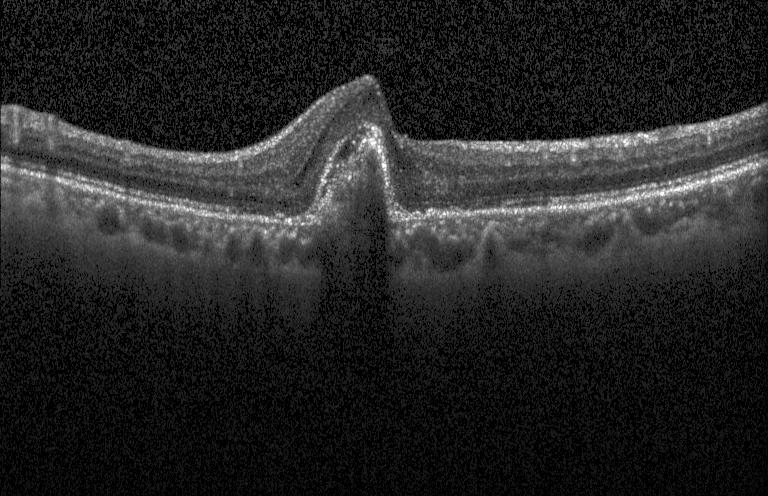
Optical coherence tomography B-scan
Assessment: a choroidal neovascular membrane.